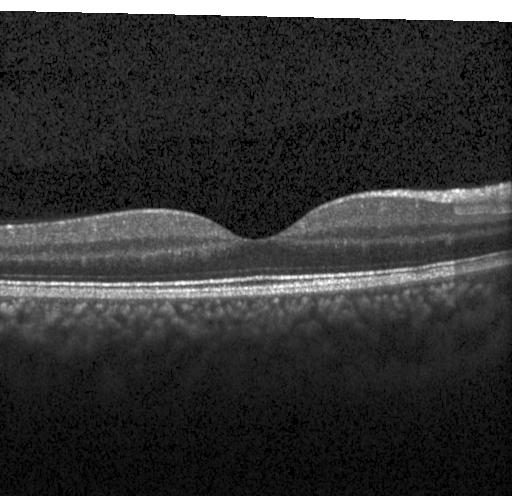 Heidelberg Spectralis; optical coherence tomography scan. This B-scan demonstrates neither CNV, DME, nor drusen.